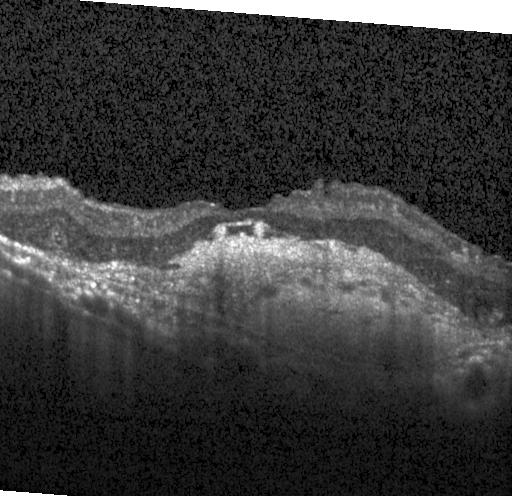 Instrument: Heidelberg Spectralis · OCT line scan.
Macular OCT: a choroidal neovascular membrane.